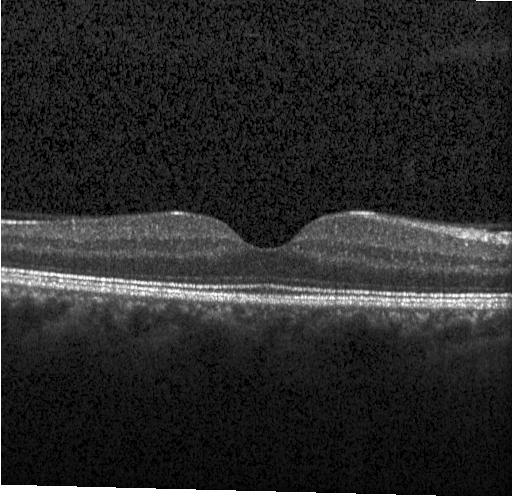
Retinal OCT cross-section
No choroidal neovascularization, no diabetic macular edema, and no drusen.